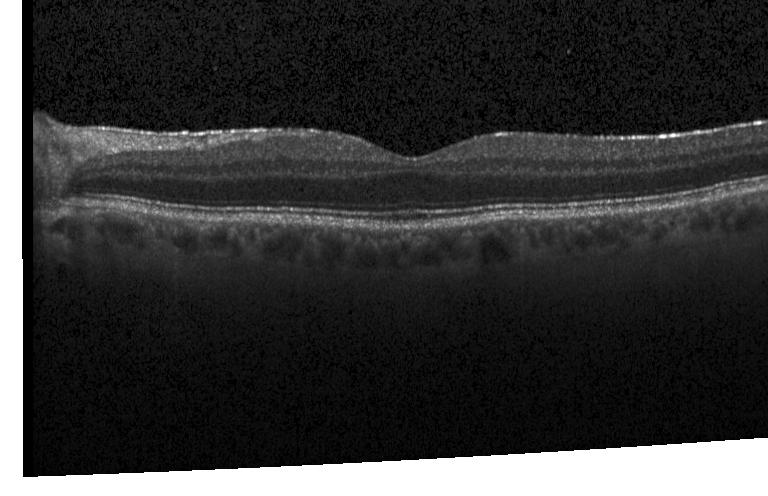
Retinal OCT B-scan — Dx: neither CNV, DME, nor drusen.